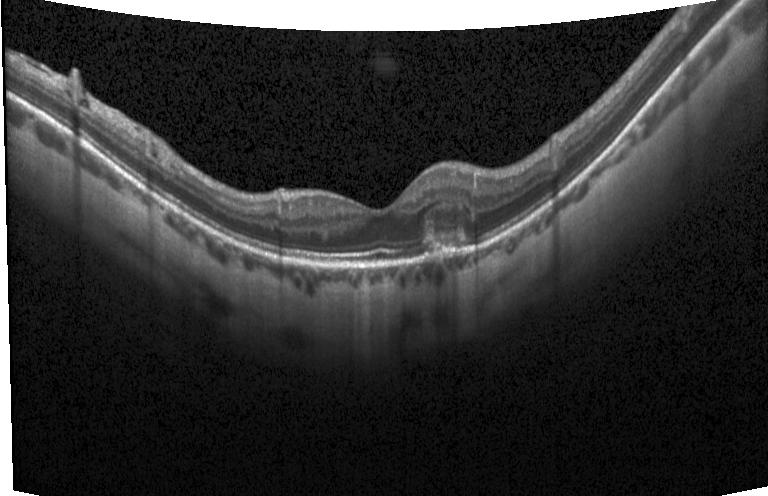

Acquired on a Heidelberg Spectralis · optical coherence tomography B-scan · centered on the fovea. Choroidal neovascularization (CNV).